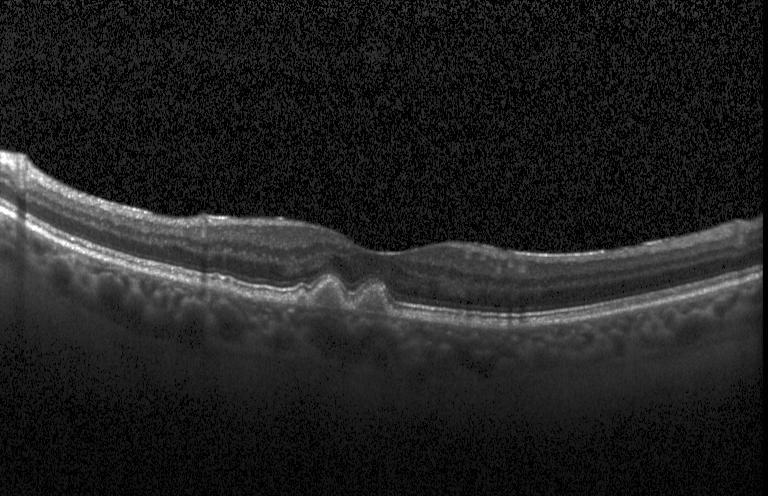

Dx: multiple drusen.